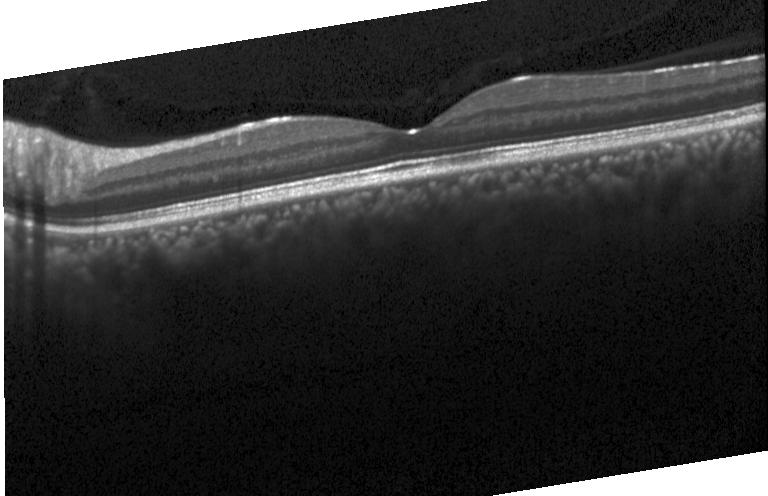

Heidelberg Spectralis OCT system. OCT line scan.
Diagnosis: no choroidal neovascularization, no diabetic macular edema, and no drusen.